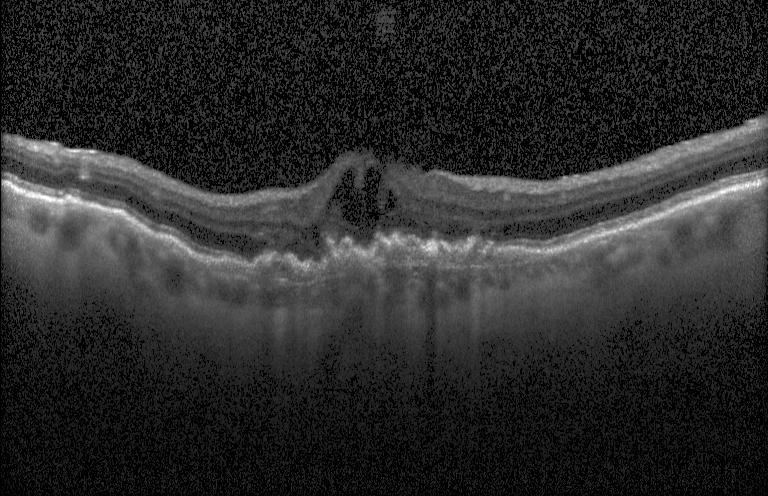
Retinal OCT cross-section — Dx: CNV.